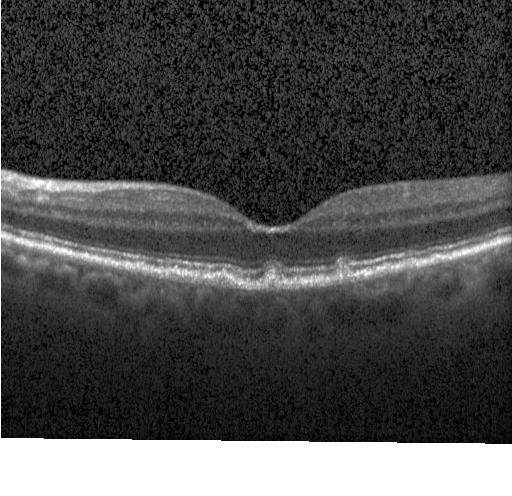 Optical coherence tomography scan
This B-scan demonstrates drusen.